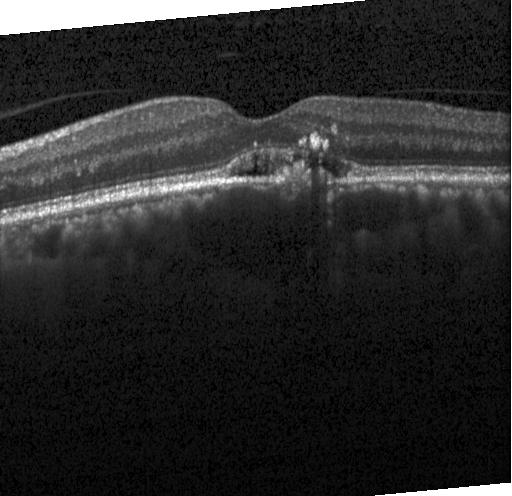 Optical coherence tomography scan — This B-scan demonstrates a choroidal neovascular membrane.